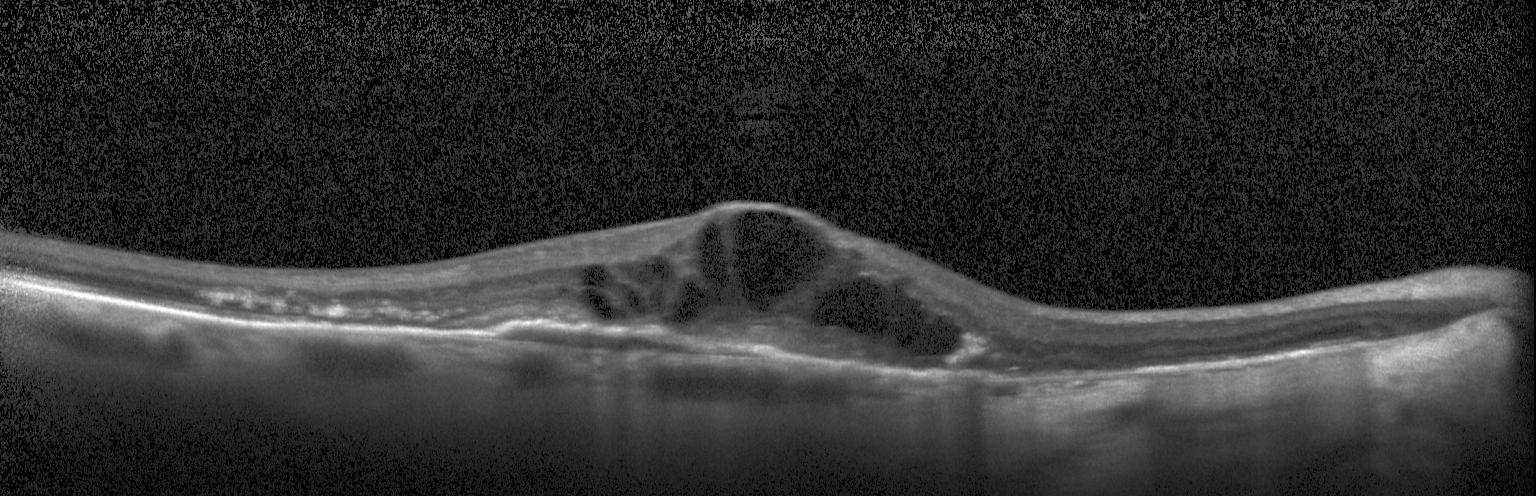
Optical coherence tomography B-scan. SD-OCT. Dx: choroidal neovascularization.